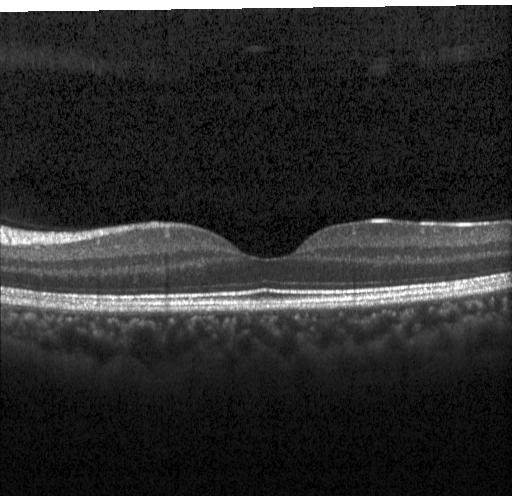
Retinal OCT B-scan, Heidelberg Spectralis. Impression: no choroidal neovascularization, no diabetic macular edema, and no drusen.